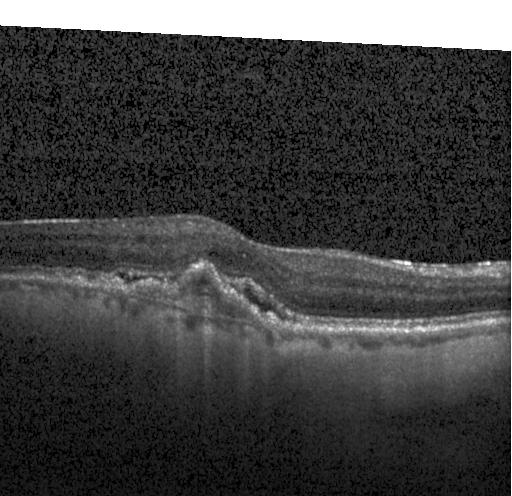

Optical coherence tomography B-scan; spectral-domain optical coherence tomography; through the macula; acquired on a Heidelberg Spectralis.
Diagnosis: a choroidal neovascular membrane.